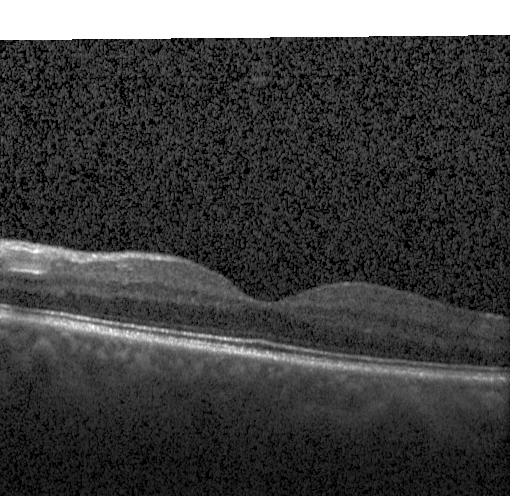
Macular scan, Heidelberg Spectralis OCT system, OCT B-scan.
Neither choroidal neovascularization, diabetic macular edema, nor drusen.